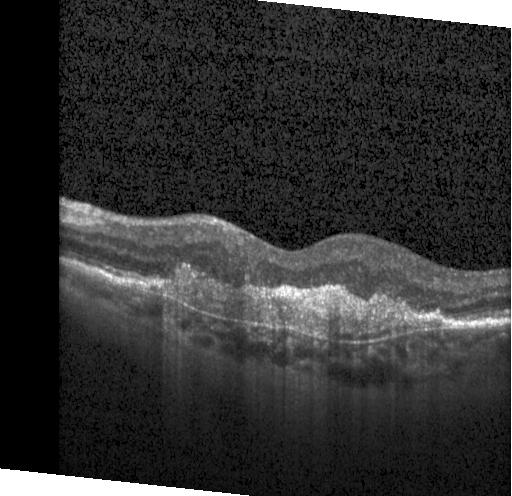

SD-OCT · fovea-centered · Heidelberg Spectralis OCT system · retinal OCT cross-section — Impression: choroidal neovascularization (CNV).